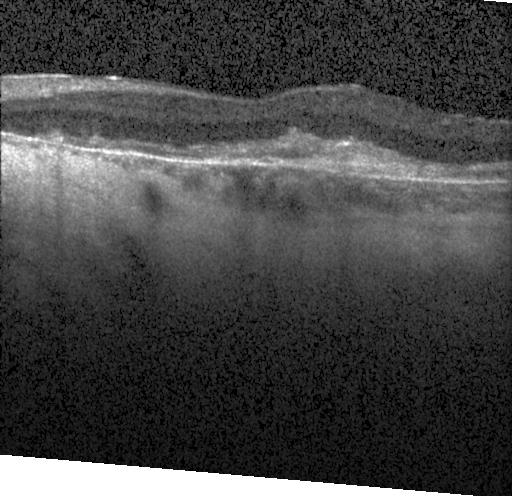 Optical coherence tomography B-scan; spectral-domain optical coherence tomography; instrument: Heidelberg Spectralis — Finding: choroidal neovascularization (CNV).